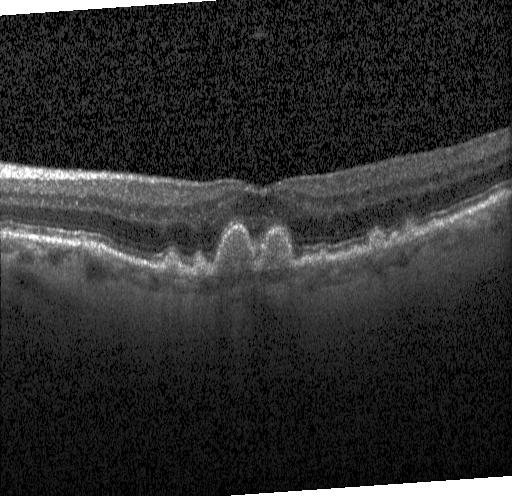
OCT B-scan. Macular OCT: multiple drusen.